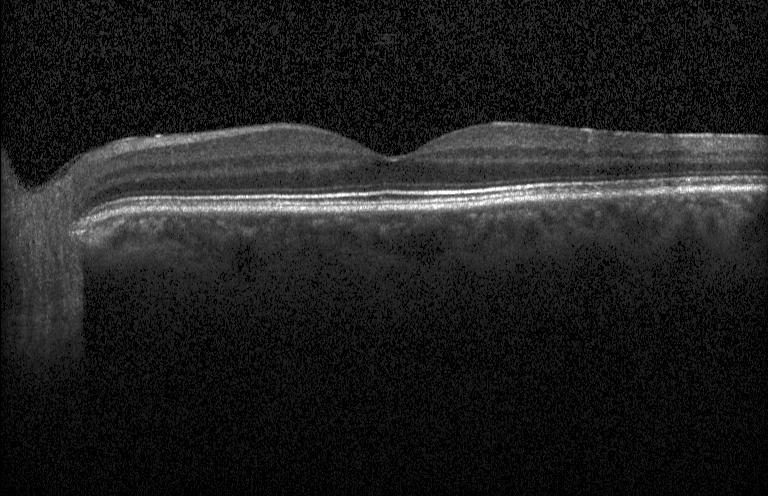

Centered on the fovea · OCT B-scan.
No evidence of choroidal neovascularization, diabetic macular edema, or drusen.